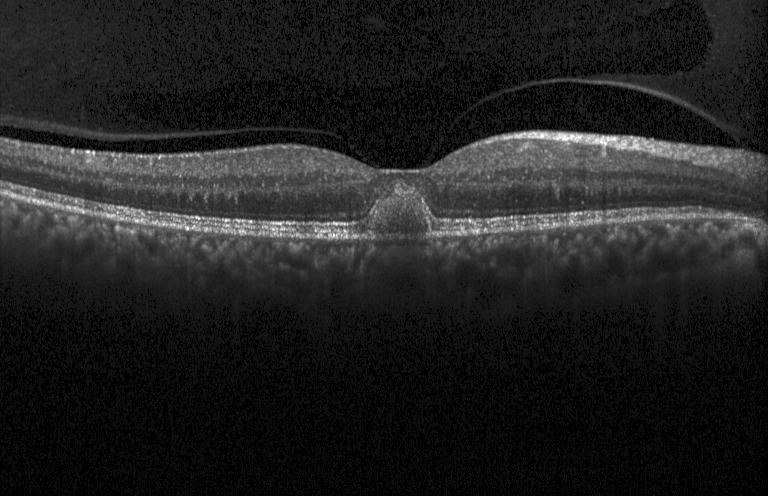 Retinal OCT B-scan. Acquired on a Heidelberg Spectralis — Impression: a choroidal neovascular membrane.